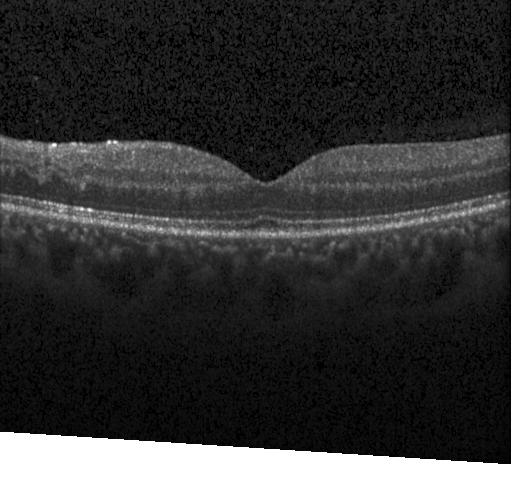

Spectral-domain optical coherence tomography · centered on the fovea · retinal OCT B-scan · acquired on a Heidelberg Spectralis
Finding: no CNV, no DME, and no drusen.